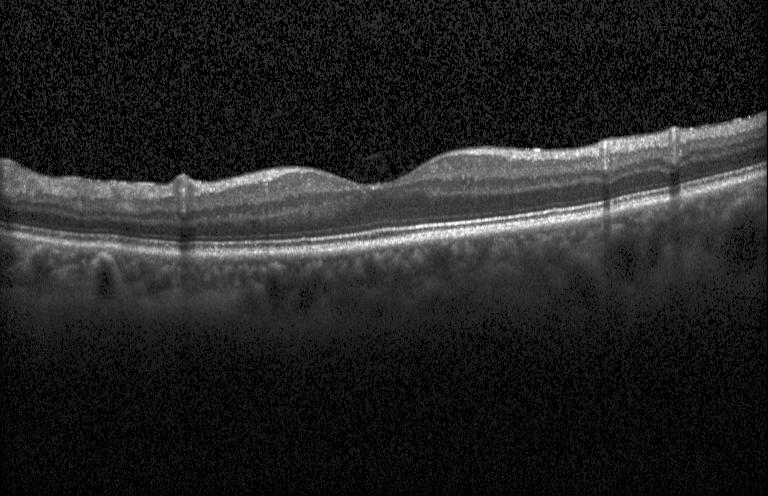
Instrument: Heidelberg Spectralis, retinal OCT cross-section — Assessment: no CNV, DME, or drusen.